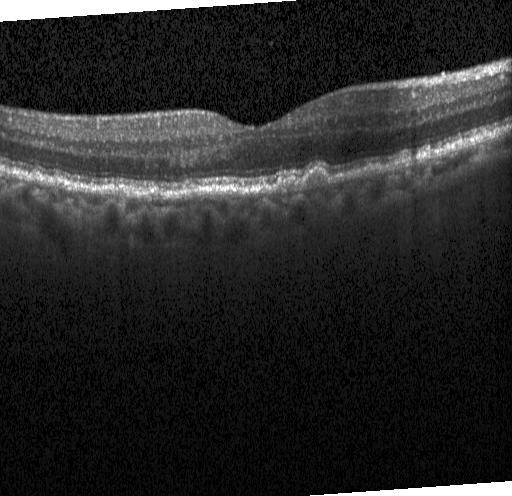 Assessment: drusen.